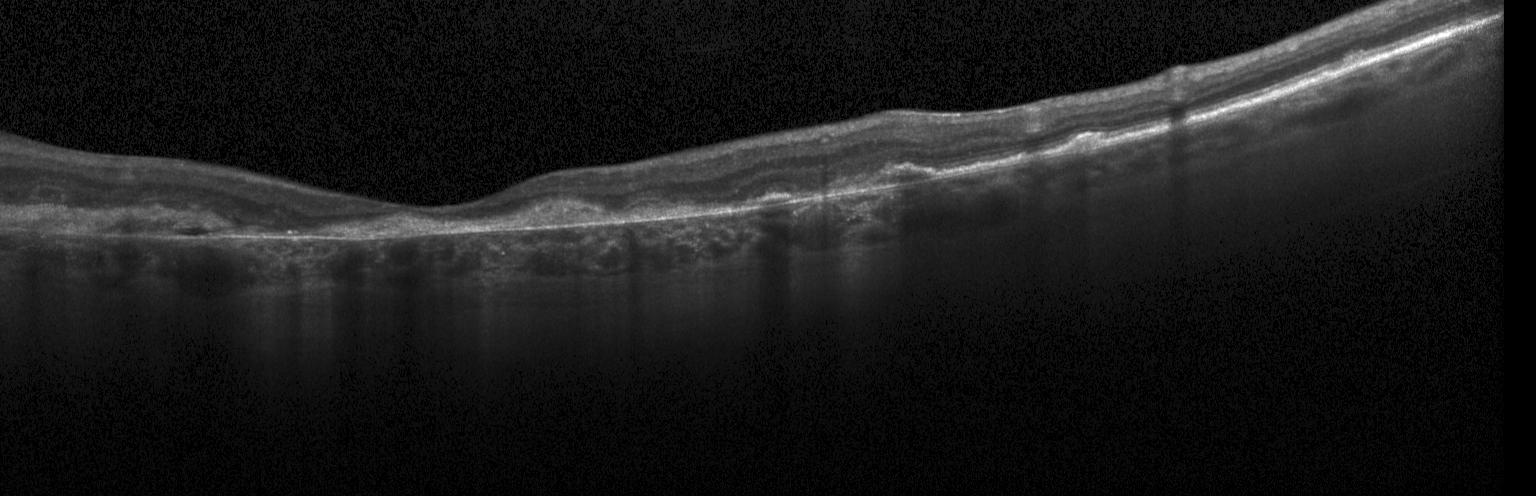
Impression: choroidal neovascularization (CNV).